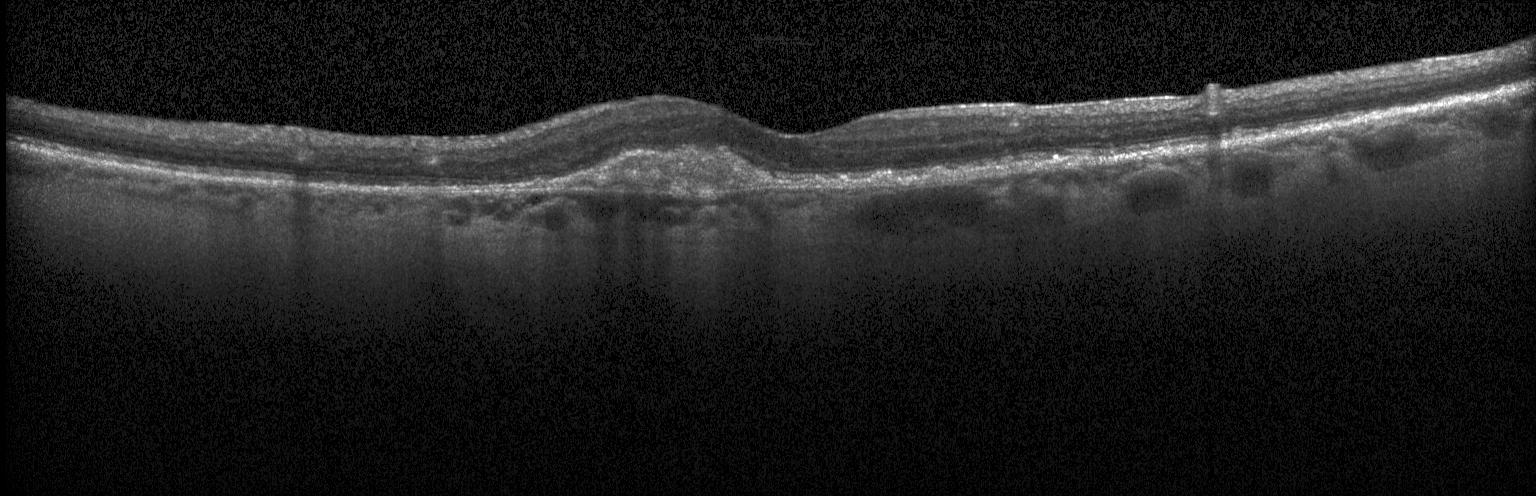 OCT B-scan. Assessment: a choroidal neovascular membrane.